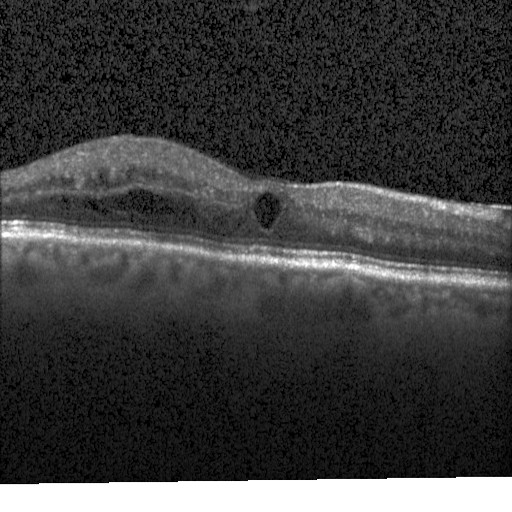

SD-OCT; horizontal scan through the fovea; OCT B-scan; acquired on a Heidelberg Spectralis. Assessment: diabetic macular edema (DME).